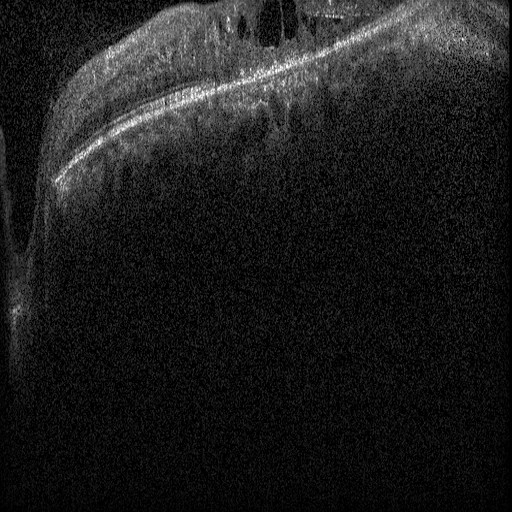 OCT line scan.
Diagnosis: diabetic macular edema (DME).